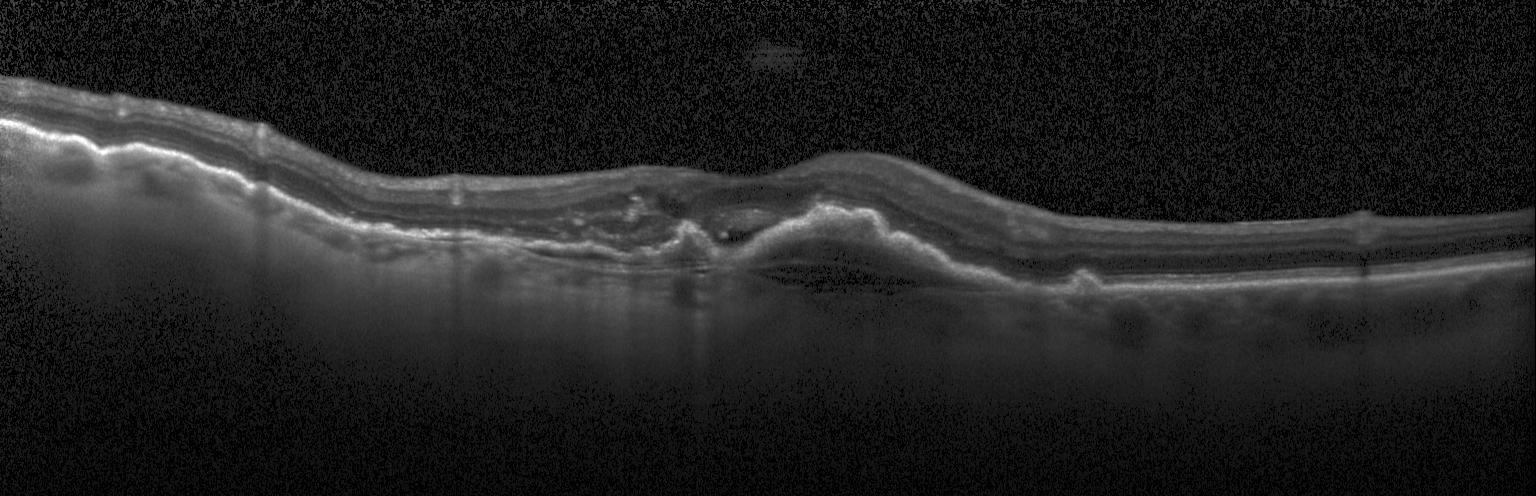 Acquired on a Heidelberg Spectralis, spectral-domain optical coherence tomography, OCT line scan, fovea-centered
Assessment: choroidal neovascularization.